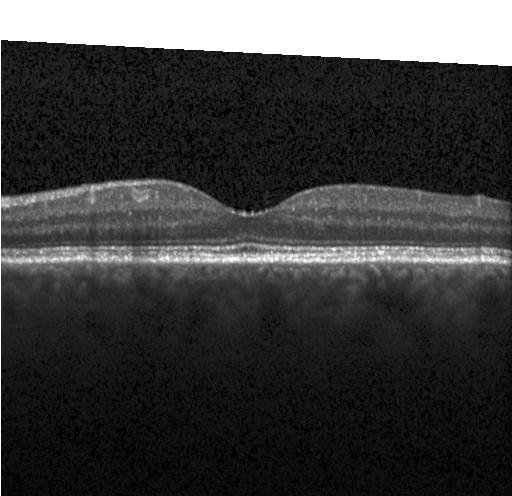 Neither choroidal neovascularization, diabetic macular edema, nor drusen.